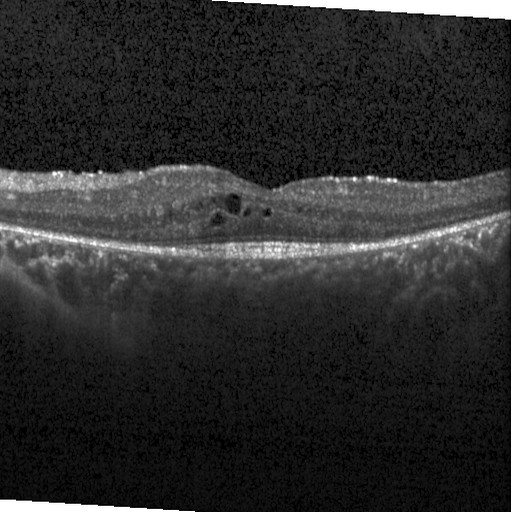

Heidelberg Spectralis OCT system · OCT line scan. Macular OCT: diabetic macular edema (DME).